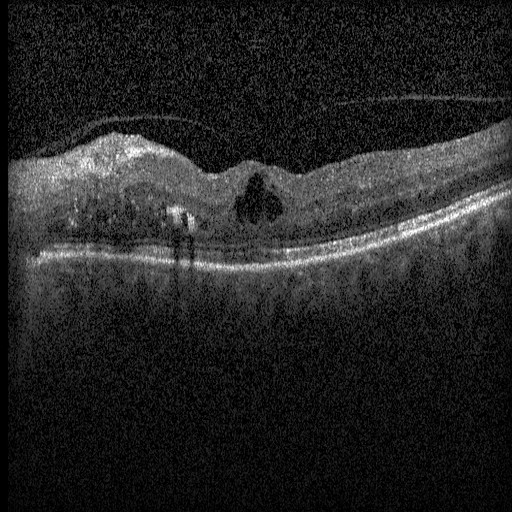
OCT B-scan, spectral-domain optical coherence tomography, centered on the fovea, Heidelberg Spectralis. OCT finding: diabetic macular edema.